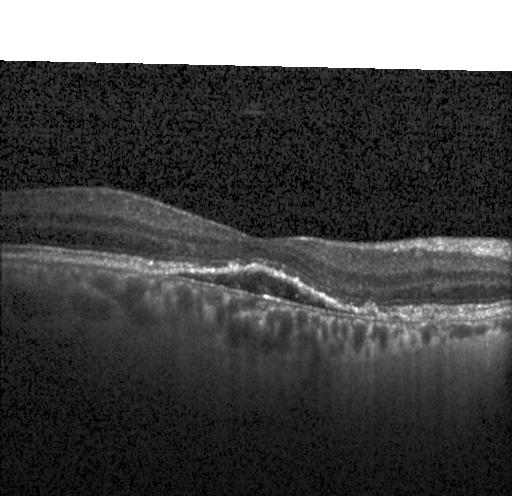
Optical coherence tomography B-scan · horizontal scan through the fovea · spectral-domain optical coherence tomography — Assessment: choroidal neovascularization.